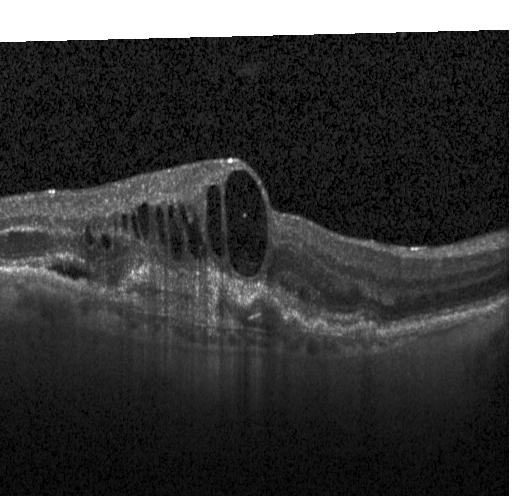

Retinal OCT cross-section
Impression: choroidal neovascularization.